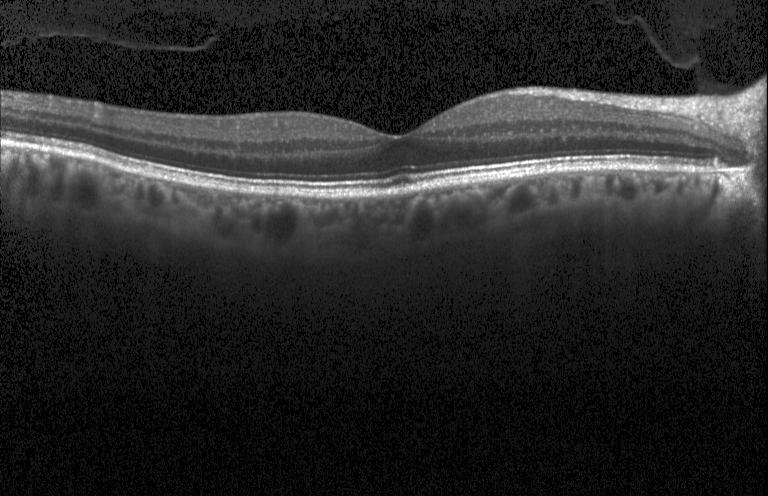
Acquired on a Heidelberg Spectralis. Spectral-domain optical coherence tomography. Retinal OCT cross-section. Horizontal scan through the fovea.
Assessment: no choroidal neovascularization, no diabetic macular edema, and no drusen.